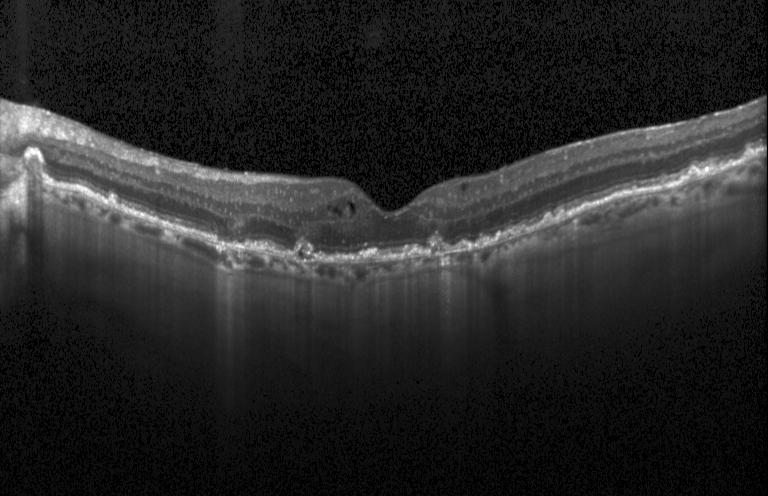 Horizontal scan through the fovea · retinal OCT cross-section · instrument: Heidelberg Spectralis. Finding: choroidal neovascularization (CNV).